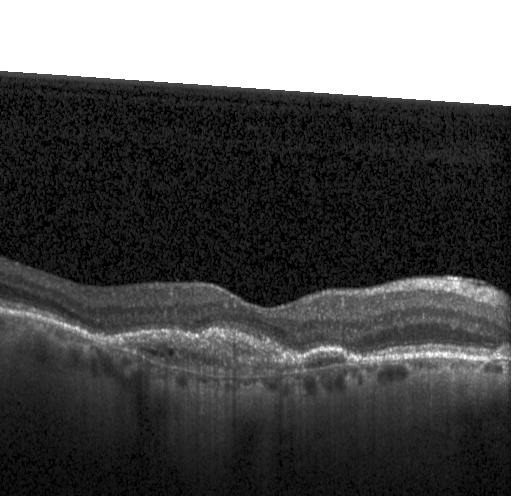 Spectral-domain optical coherence tomography. Heidelberg Spectralis. Optical coherence tomography scan — Choroidal neovascularization (CNV).